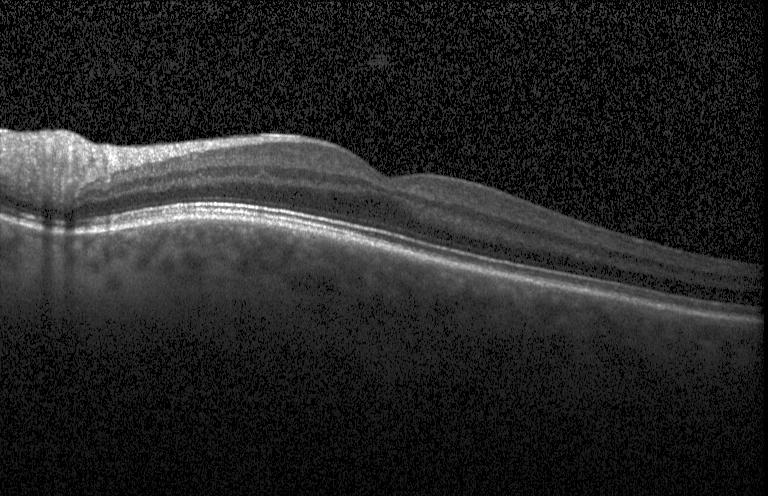

Optical coherence tomography scan, spectral-domain OCT.
Impression: no evidence of CNV, DME, or drusen.